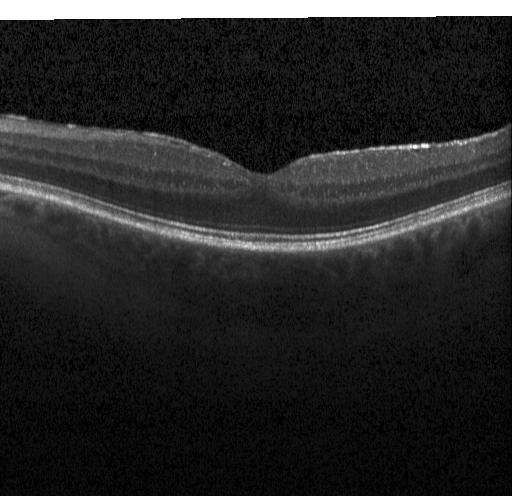

Retinal OCT cross-section
Finding: no evidence of choroidal neovascularization, diabetic macular edema, or drusen.